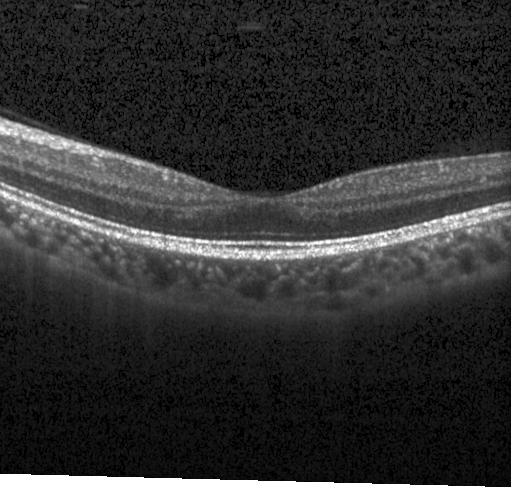

Spectral-domain OCT. Retinal OCT cross-section. Horizontal scan through the fovea. Acquired on a Heidelberg Spectralis
Diagnosis: neither CNV, DME, nor drusen.